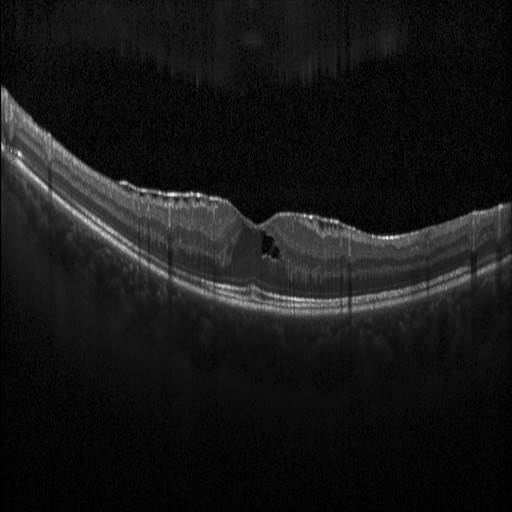

OCT B-scan
Diagnosis: diabetic macular edema (DME).